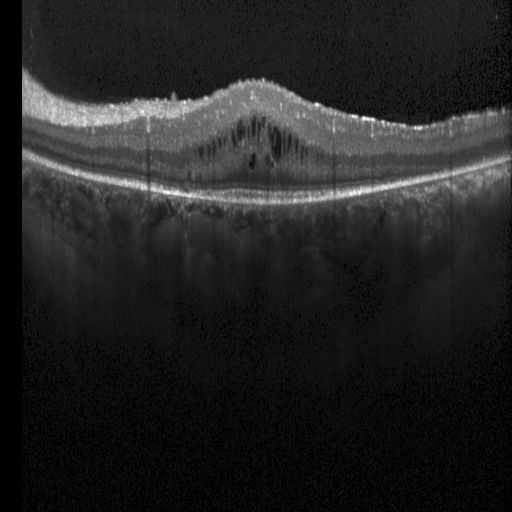

Dx: diabetic macular edema (DME).